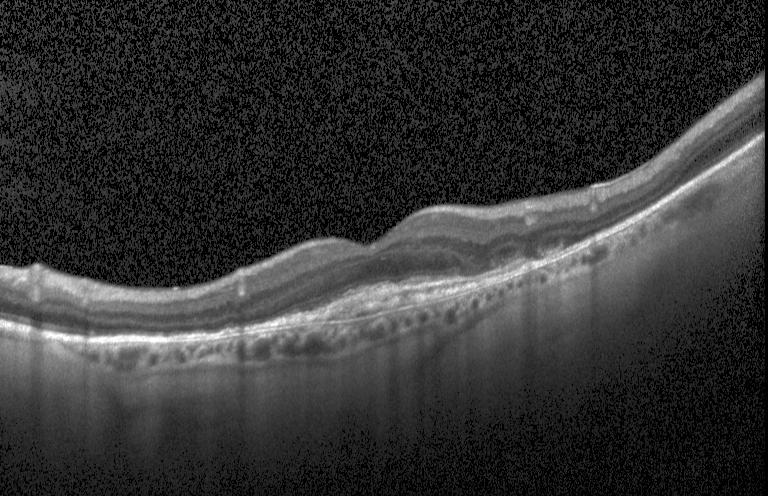
Spectral-domain optical coherence tomography. OCT B-scan. Instrument: Heidelberg Spectralis. Macular scan — Impression: a choroidal neovascular membrane.